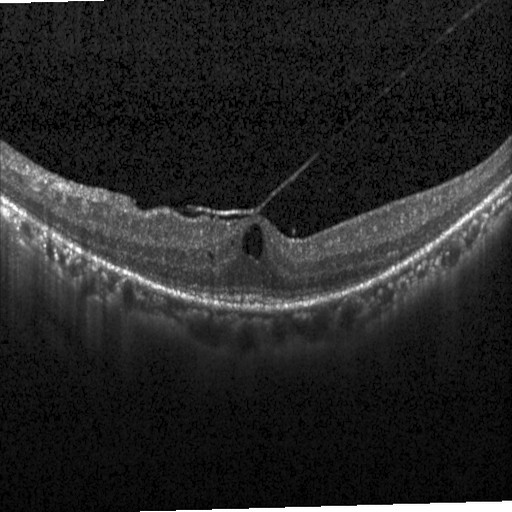 Diagnosis: DME.